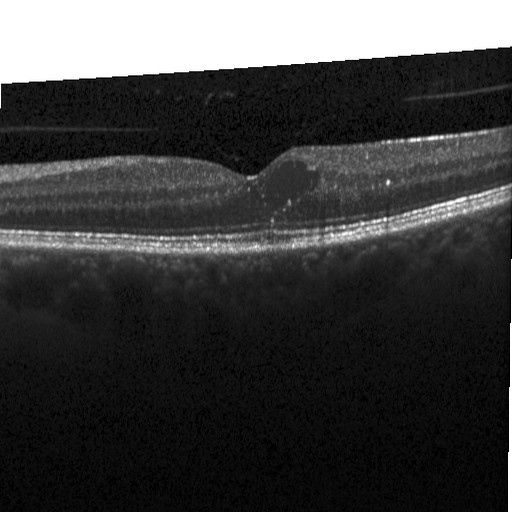 Spectral-domain OCT · through the macula · Heidelberg Spectralis · OCT line scan. This B-scan demonstrates DME.